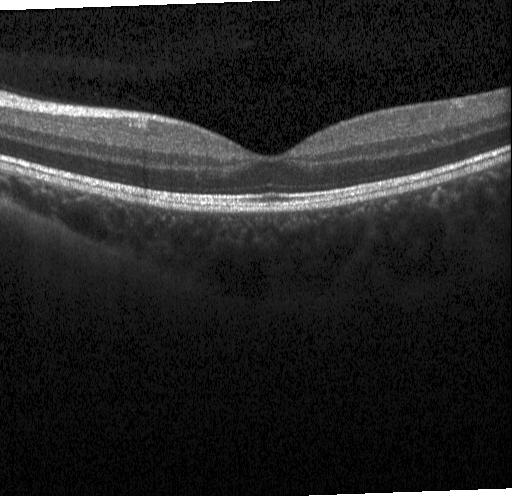 Diagnosis: no evidence of CNV, DME, or drusen.